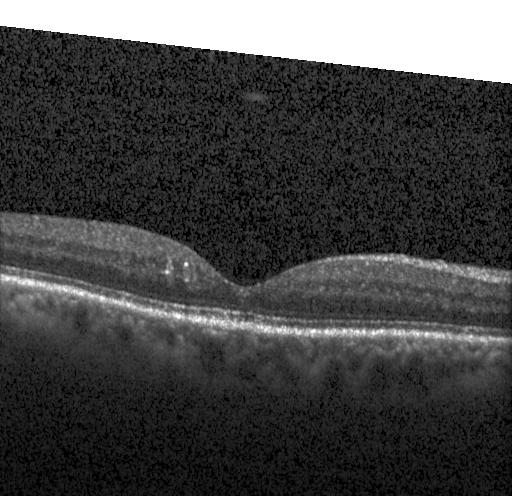

Retinal OCT cross-section.
OCT finding: no evidence of CNV, DME, or drusen.